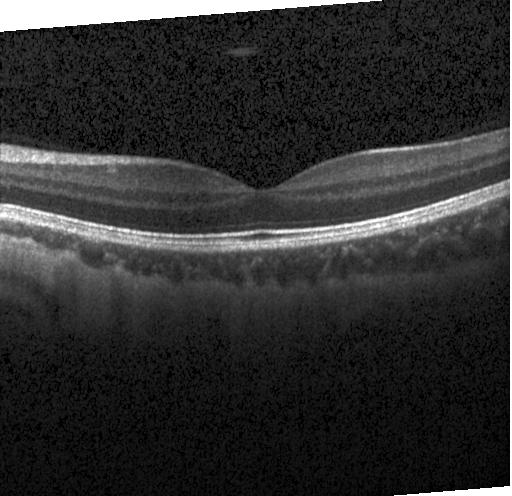

Finding: no evidence of CNV, DME, or drusen.